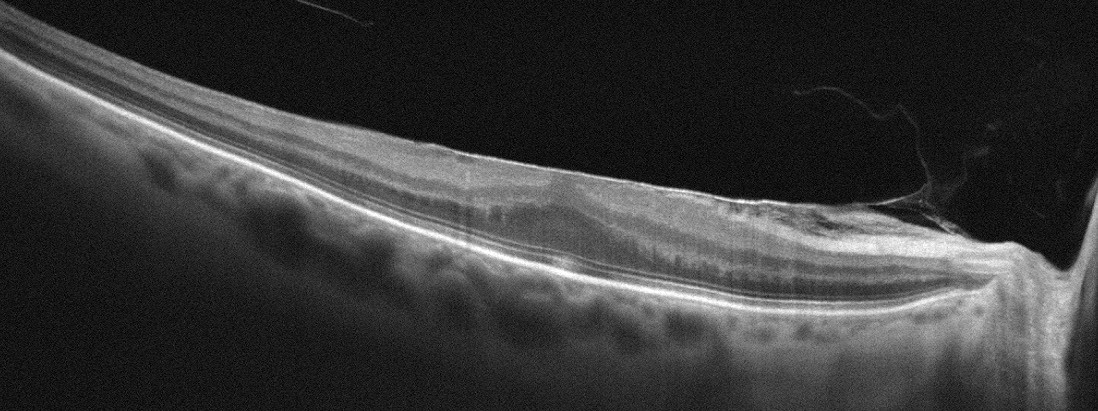
Retinal OCT cross-section
OCT finding: epiretinal membrane.